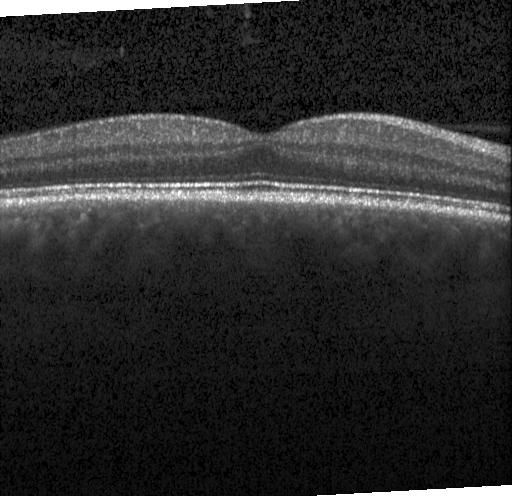

Macular OCT: no choroidal neovascularization, no diabetic macular edema, and no drusen.